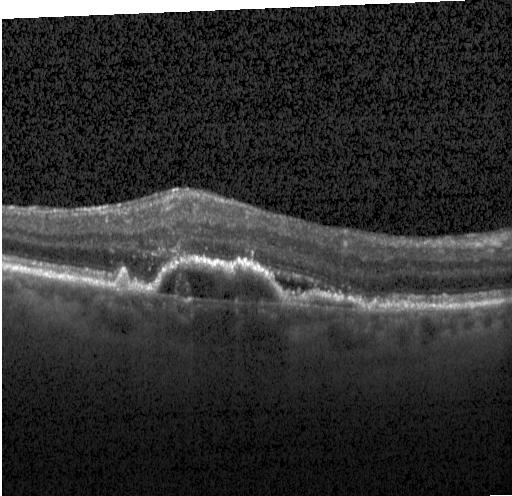 Retinal OCT cross-section — Assessment: a choroidal neovascular membrane.